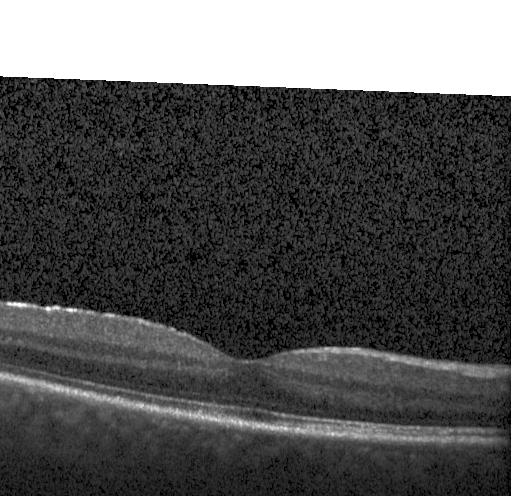 Through the macula. Retinal OCT B-scan. SD-OCT. Dx: no choroidal neovascularization, diabetic macular edema, or drusen.